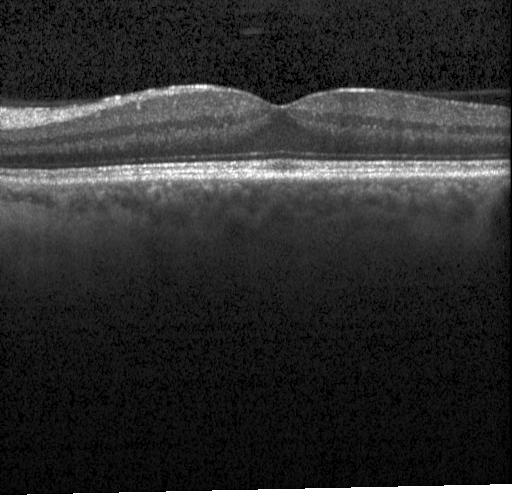 Optical coherence tomography scan. Heidelberg Spectralis OCT system. Macular scan. Spectral-domain OCT. OCT finding: neither choroidal neovascularization, diabetic macular edema, nor drusen.